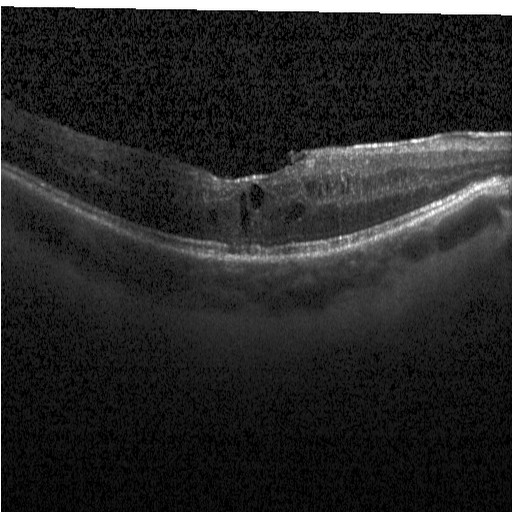
Diagnosis: DME.